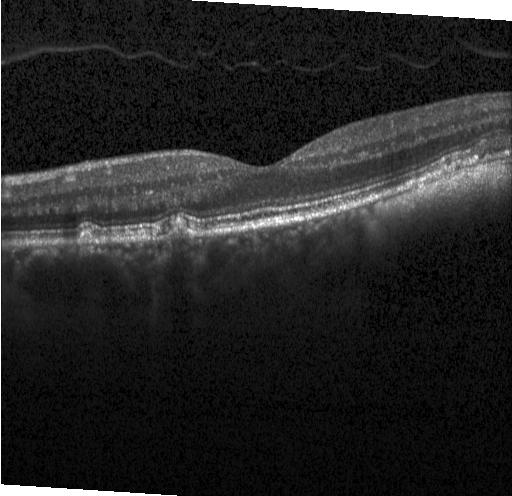

Finding: multiple drusen.